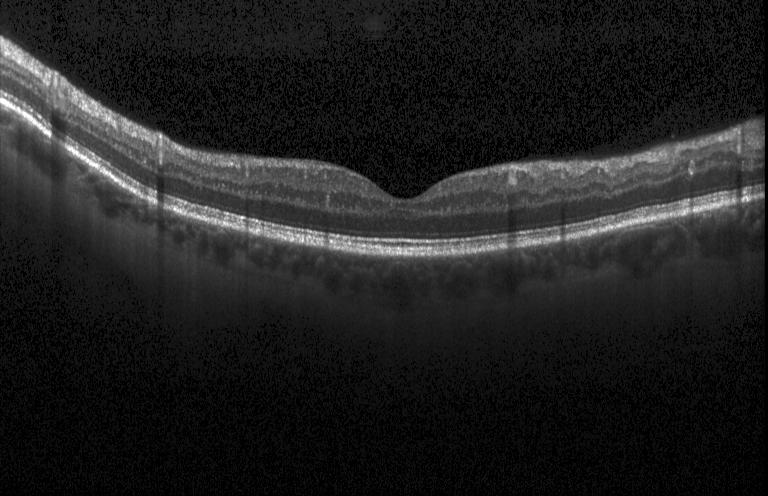 Finding: no choroidal neovascularization, no diabetic macular edema, and no drusen.